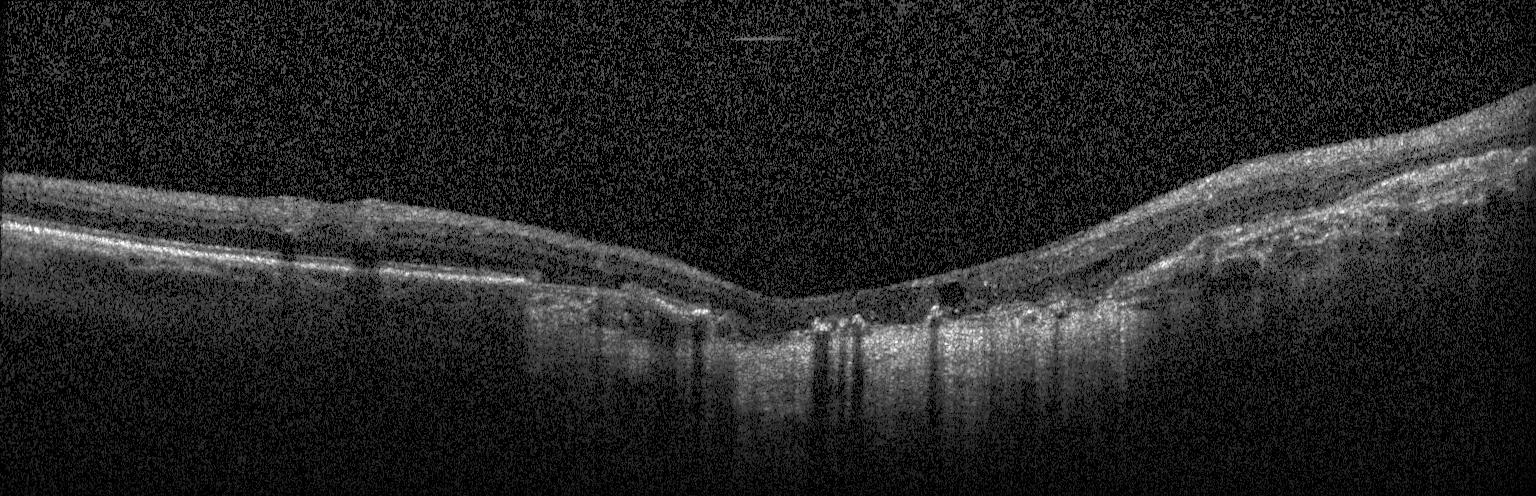 Spectral-domain optical coherence tomography · Heidelberg Spectralis · horizontal scan through the fovea · retinal OCT B-scan
Dx: a choroidal neovascular membrane.